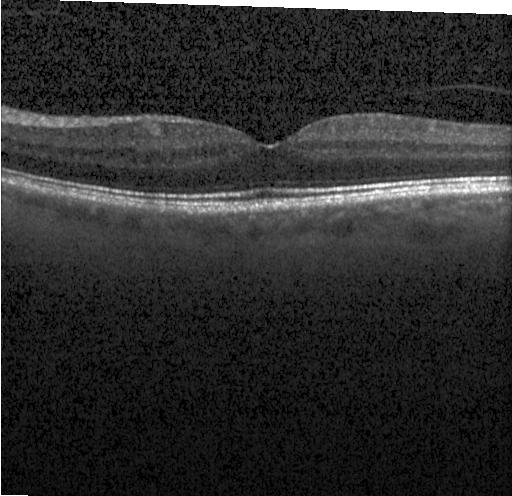 Optical coherence tomography scan, horizontal scan through the fovea, Heidelberg Spectralis — Macular OCT: no evidence of choroidal neovascularization, diabetic macular edema, or drusen.